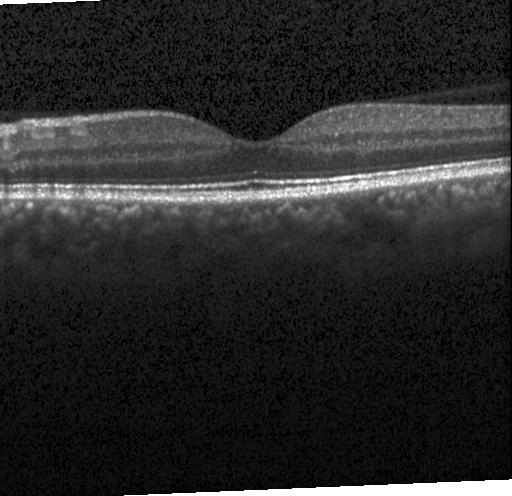 Neither choroidal neovascularization, diabetic macular edema, nor drusen.